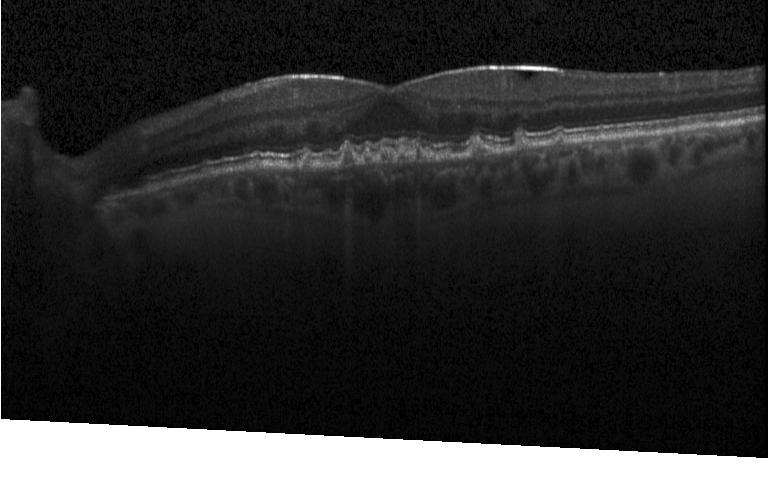 Optical coherence tomography B-scan — This B-scan demonstrates drusen.